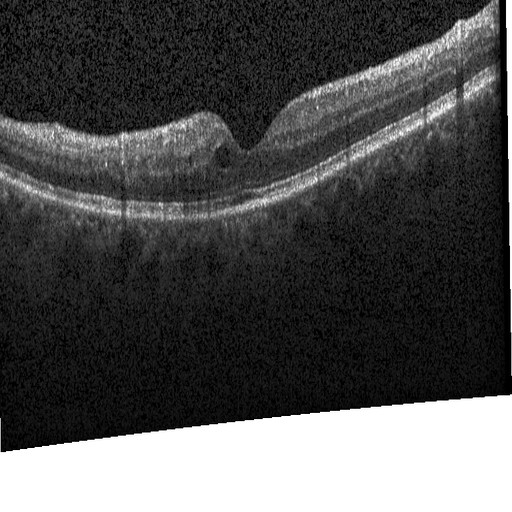 Diagnosis: diabetic macular edema (DME).